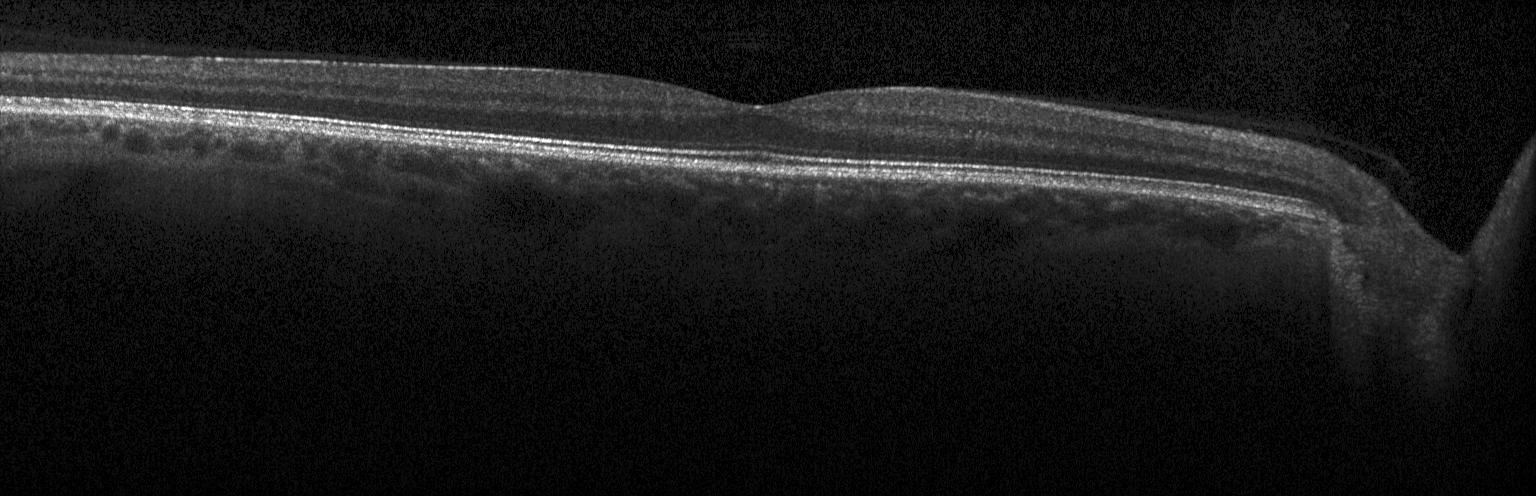

Diagnosis: no CNV, no DME, and no drusen.